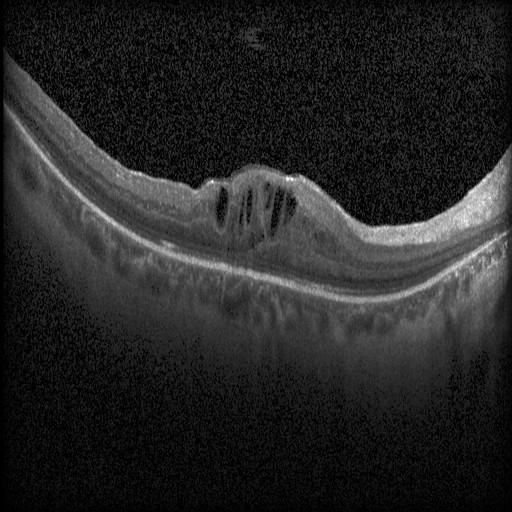

OCT B-scan, SD-OCT, fovea-centered, instrument: Heidelberg Spectralis.
OCT finding: DME.